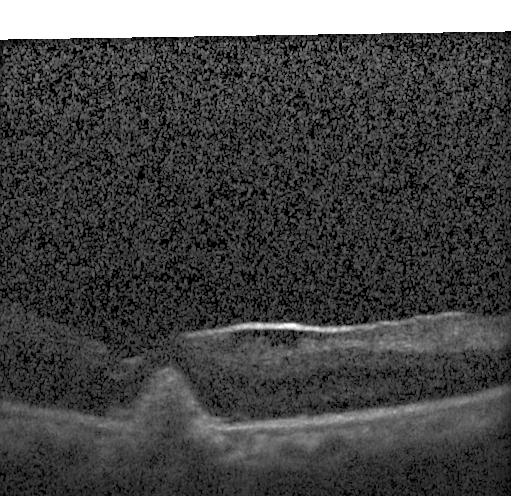 SD-OCT · fovea-centered · optical coherence tomography scan — Diagnosis: a choroidal neovascular membrane.